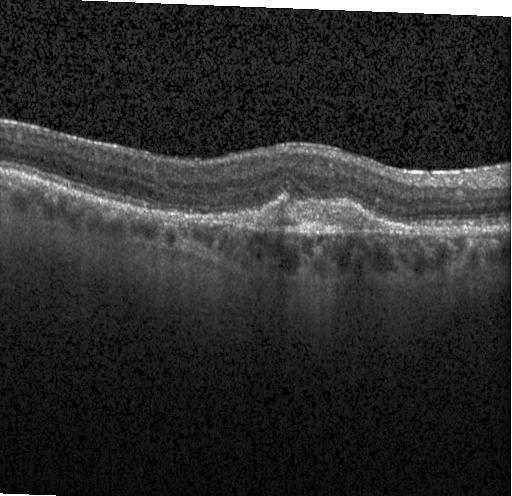 This B-scan demonstrates a choroidal neovascular membrane.